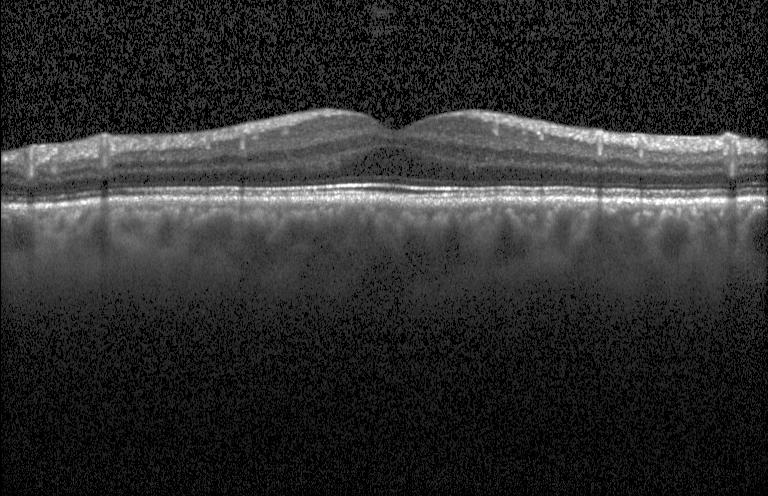 Dx: no CNV, no DME, and no drusen.